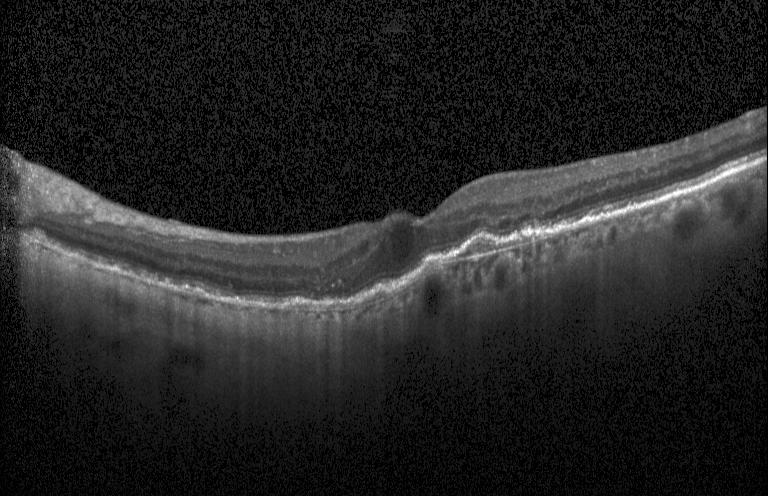
Dx: choroidal neovascularization (CNV).